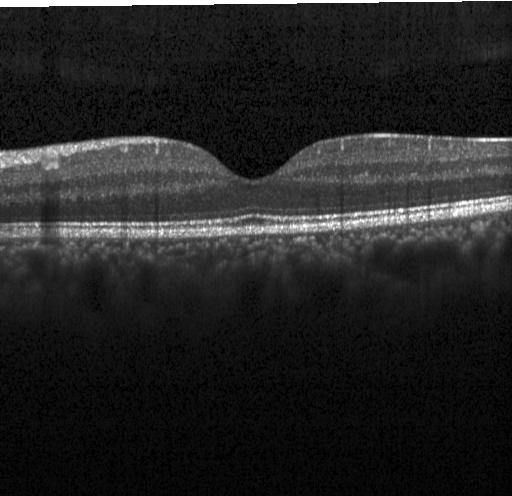 Acquired on a Heidelberg Spectralis · optical coherence tomography scan — Diagnosis: neither choroidal neovascularization, diabetic macular edema, nor drusen.